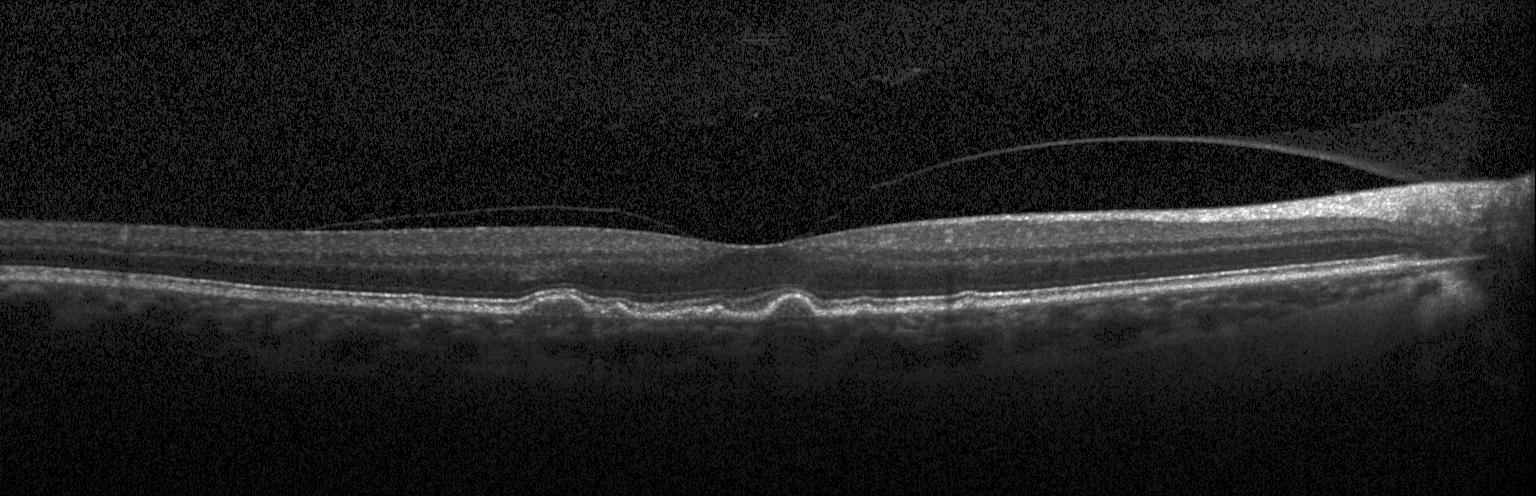
OCT line scan; spectral-domain optical coherence tomography; through the macula
Multiple drusen.